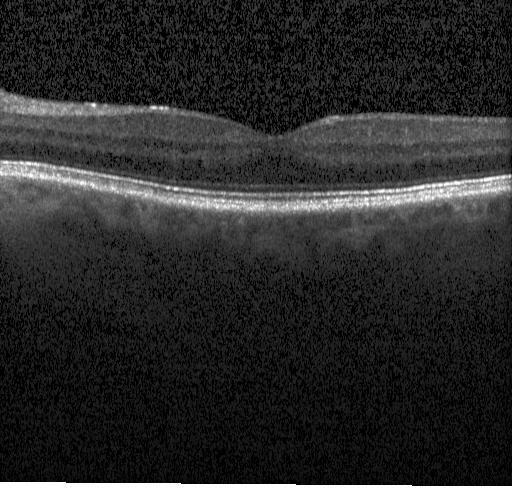
Optical coherence tomography scan. Spectral-domain optical coherence tomography
The scan shows no choroidal neovascularization, diabetic macular edema, or drusen.